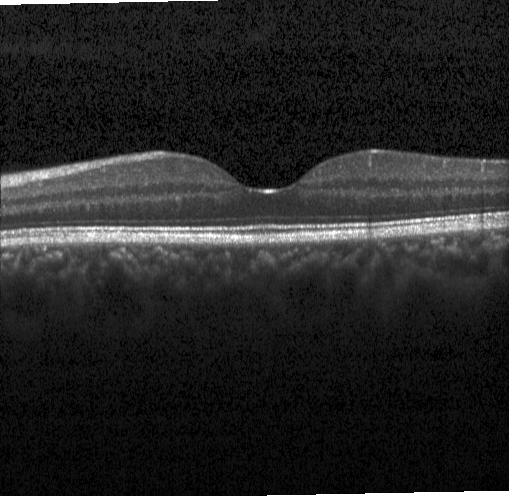
This B-scan demonstrates no choroidal neovascularization, diabetic macular edema, or drusen.